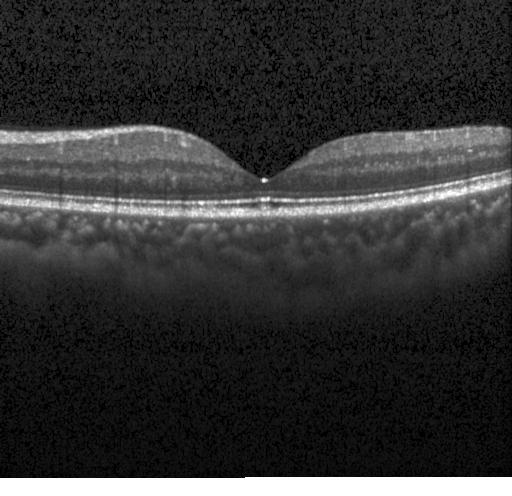 Diagnosis: no choroidal neovascularization, no diabetic macular edema, and no drusen.